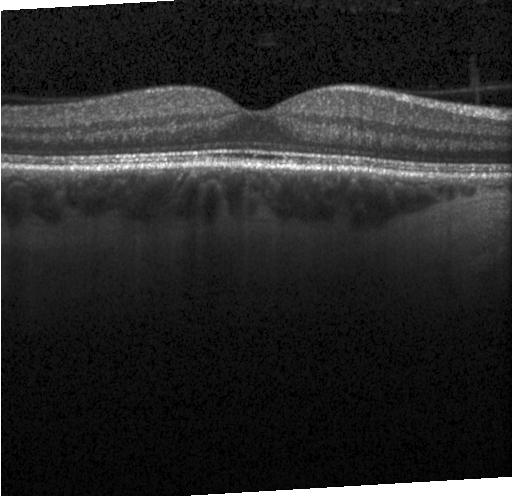
Retinal OCT cross-section showing no choroidal neovascularization, diabetic macular edema, or drusen.